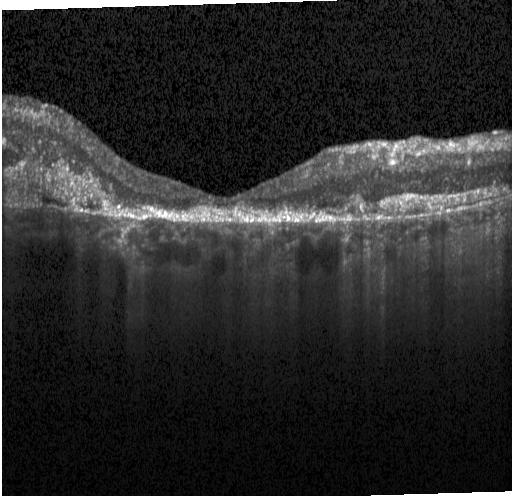

Spectral-domain OCT · Heidelberg Spectralis OCT system · OCT line scan · centered on the fovea. A choroidal neovascular membrane.